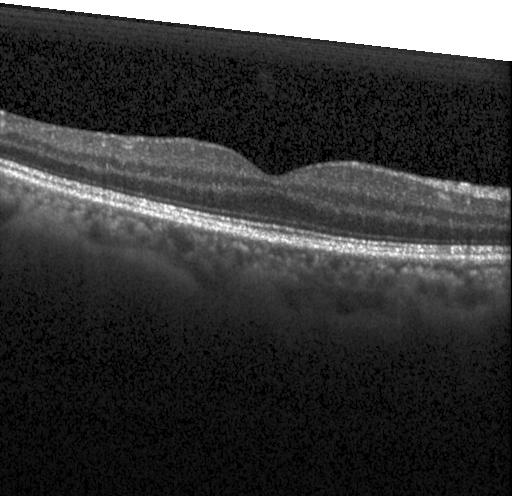

SD-OCT; OCT line scan — Assessment: no choroidal neovascularization, no diabetic macular edema, and no drusen.